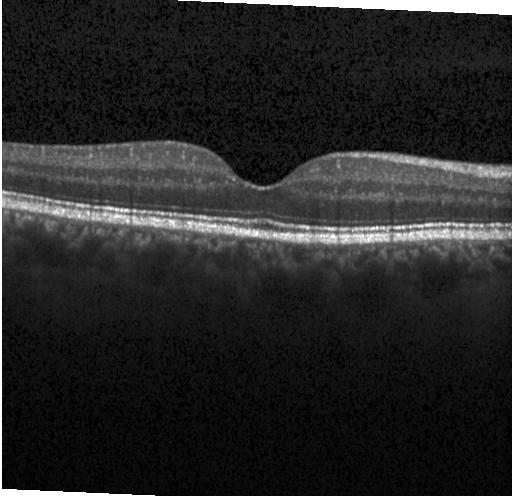

Heidelberg Spectralis OCT system · spectral-domain OCT · retinal OCT cross-section · macular scan.
No CNV, no DME, and no drusen.